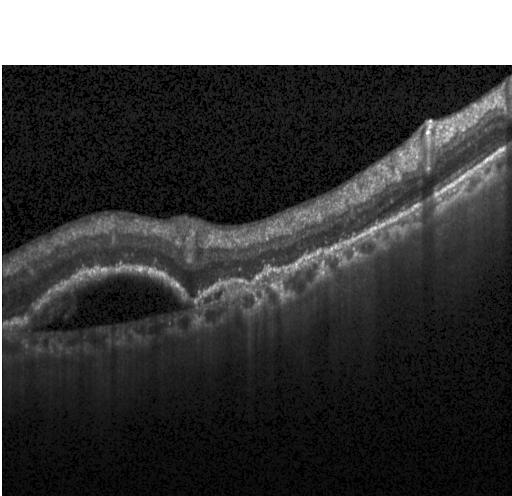

SD-OCT; optical coherence tomography B-scan; Heidelberg Spectralis; macular scan.
OCT finding: CNV.